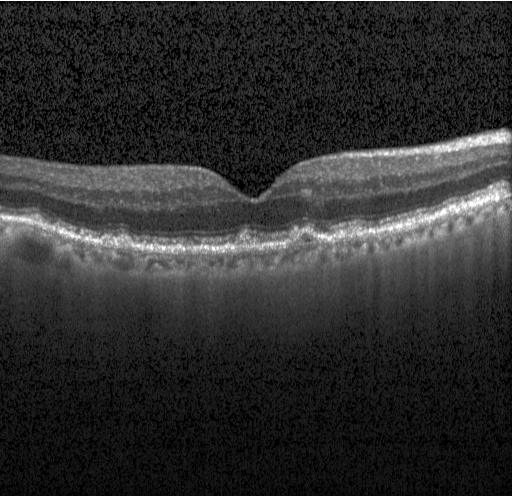
Centered on the fovea; OCT B-scan
Impression: drusen.